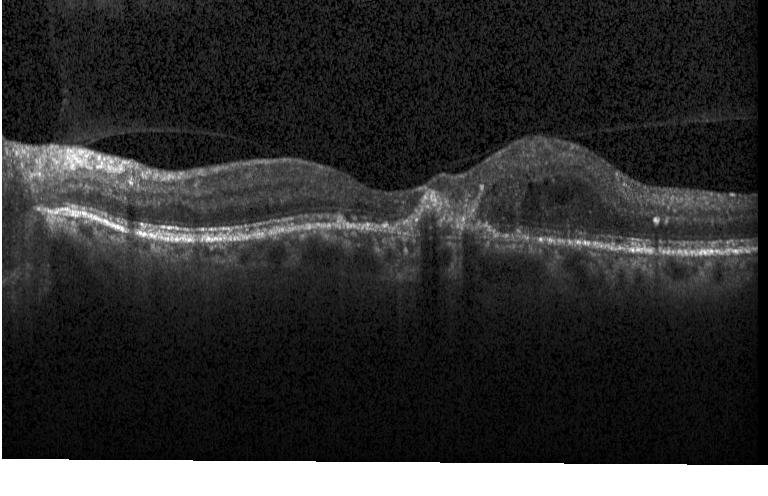
Horizontal scan through the fovea. OCT B-scan. SD-OCT
Diagnosis: a choroidal neovascular membrane.